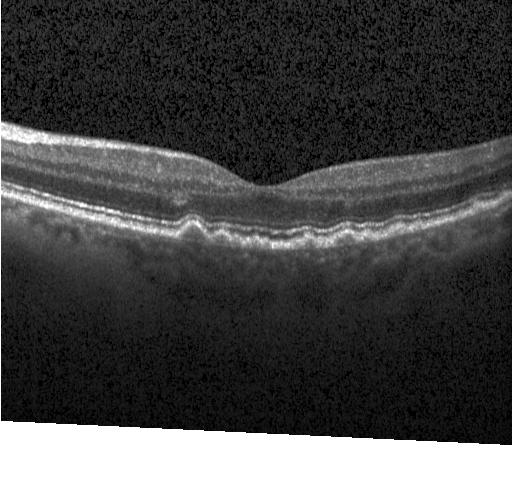
OCT scan showing drusen.